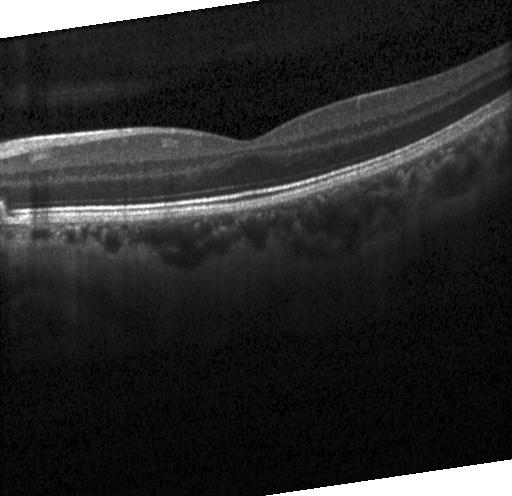
Macular scan; optical coherence tomography B-scan.
OCT finding: no CNV, no DME, and no drusen.